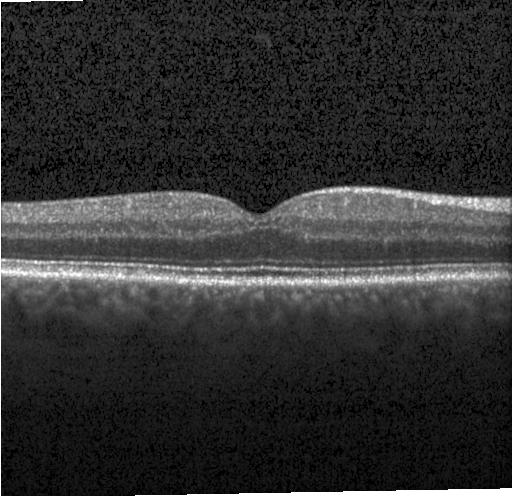 Retinal OCT B-scan, SD-OCT, macular scan
Finding: no evidence of choroidal neovascularization, diabetic macular edema, or drusen.